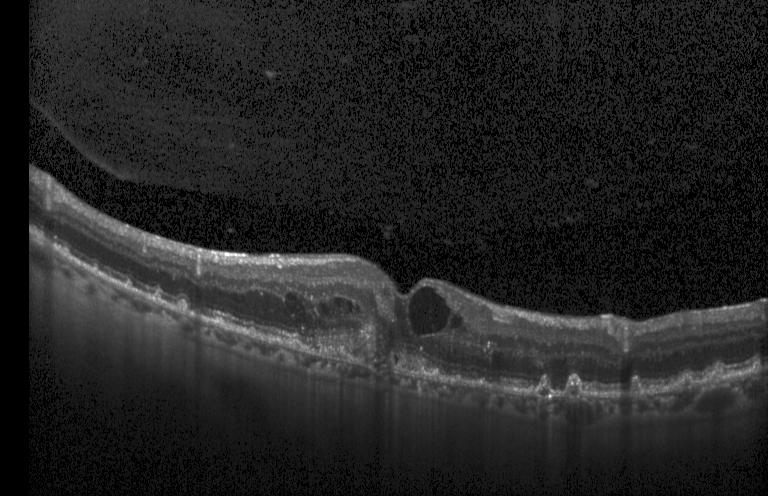
OCT finding: a choroidal neovascular membrane.